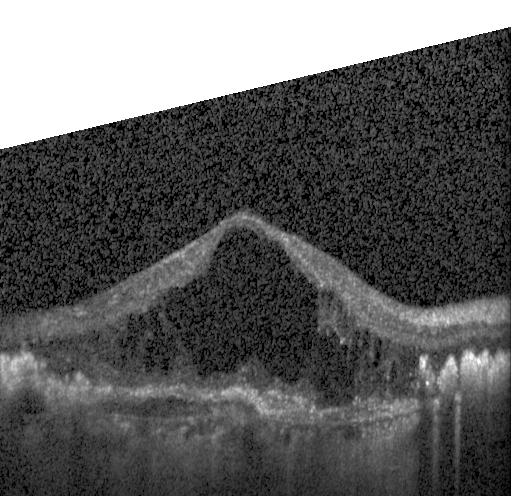

Centered on the fovea, spectral-domain optical coherence tomography, OCT line scan — Diagnosis: a choroidal neovascular membrane.